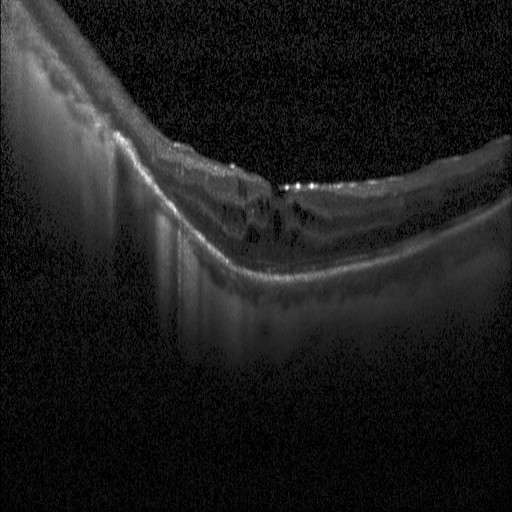 Diagnosis: DME.